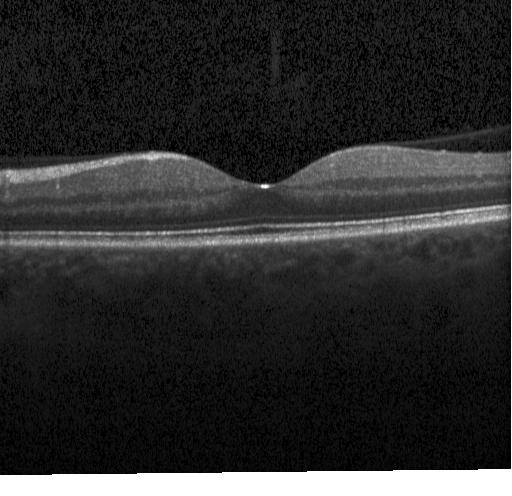
Retinal OCT cross-section.
Finding: no choroidal neovascularization, diabetic macular edema, or drusen.